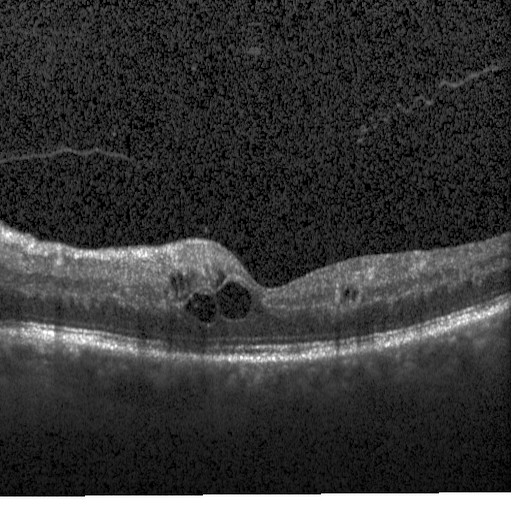 Instrument: Heidelberg Spectralis; spectral-domain OCT; through the macula; OCT line scan — DME.